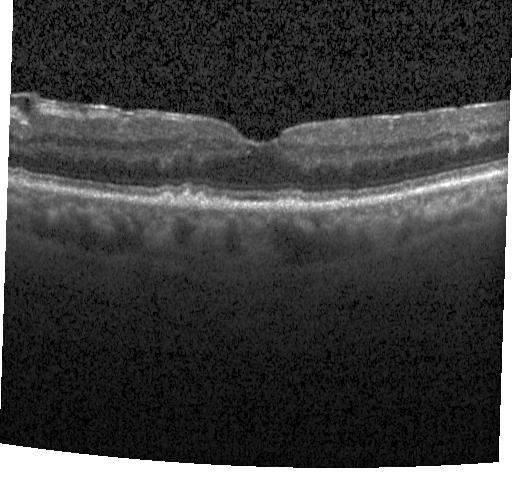 Dx: sub-RPE drusenoid deposits.